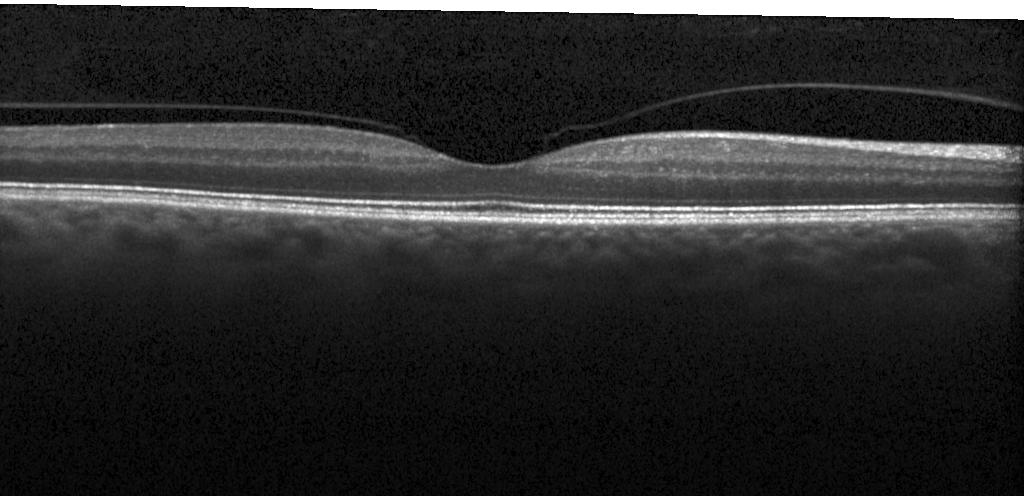
Retinal OCT B-scan. Finding: no evidence of choroidal neovascularization, diabetic macular edema, or drusen.